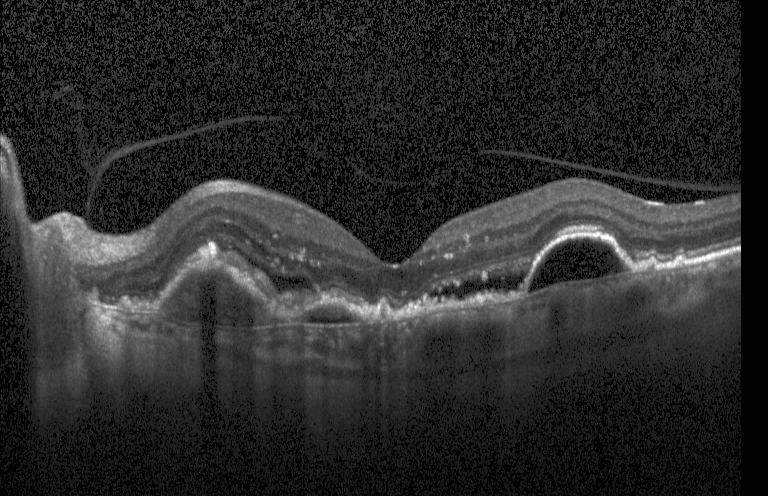 Spectral-domain optical coherence tomography · retinal OCT B-scan · horizontal scan through the fovea.
This B-scan demonstrates a choroidal neovascular membrane.